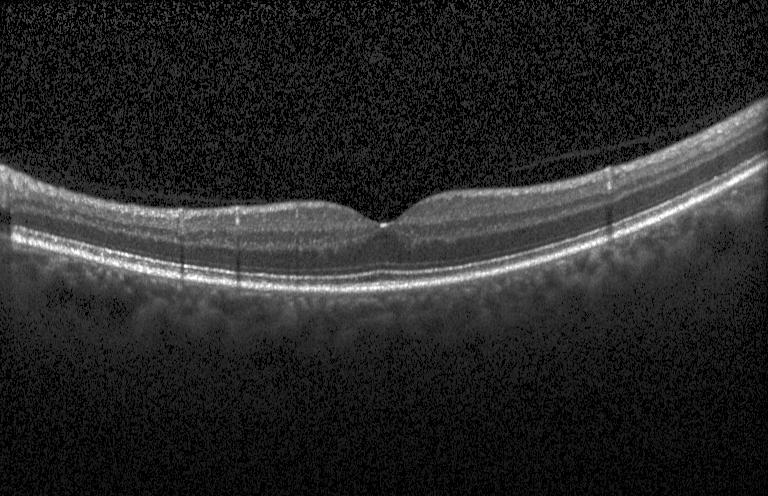 Diagnosis: neither CNV, DME, nor drusen.